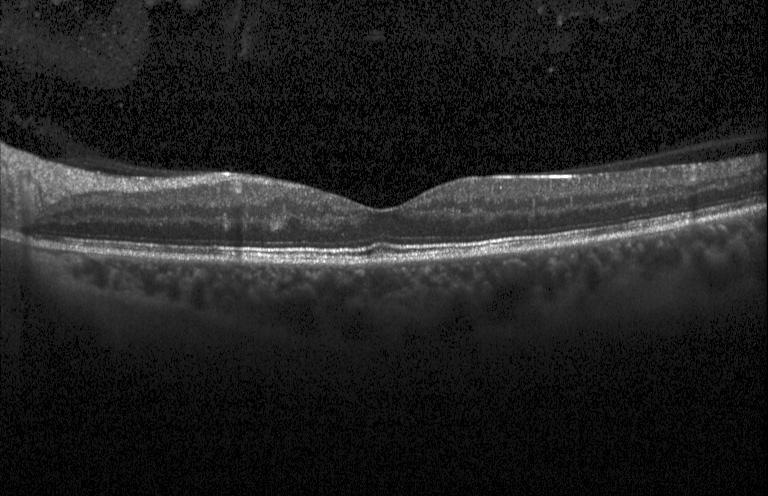
Instrument: Heidelberg Spectralis · optical coherence tomography scan.
Dx: no choroidal neovascularization, diabetic macular edema, or drusen.